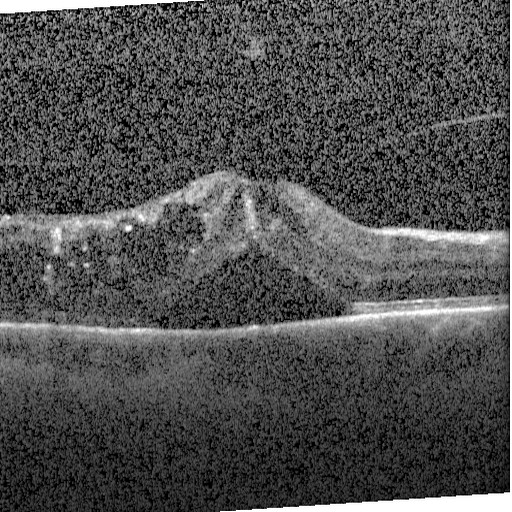

OCT scan showing DME.